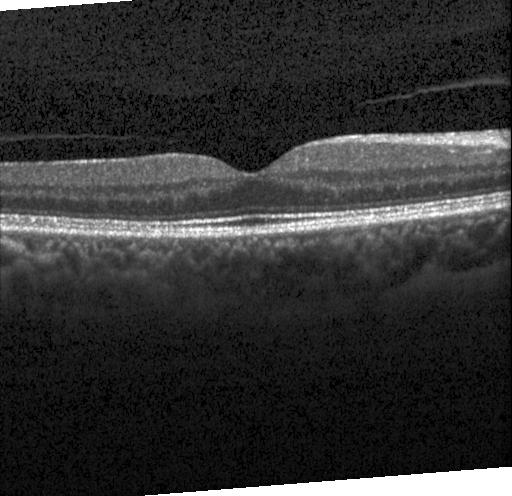
Finding: no CNV, DME, or drusen.